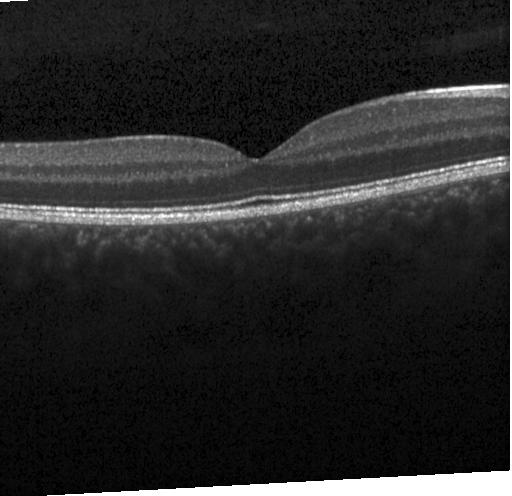 OCT B-scan showing no choroidal neovascularization, no diabetic macular edema, and no drusen.